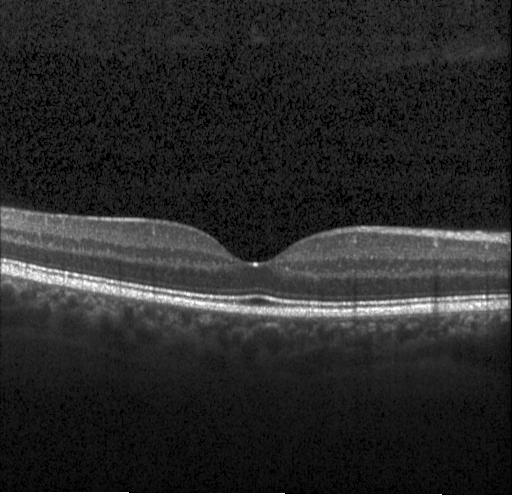

Dx: neither choroidal neovascularization, diabetic macular edema, nor drusen.